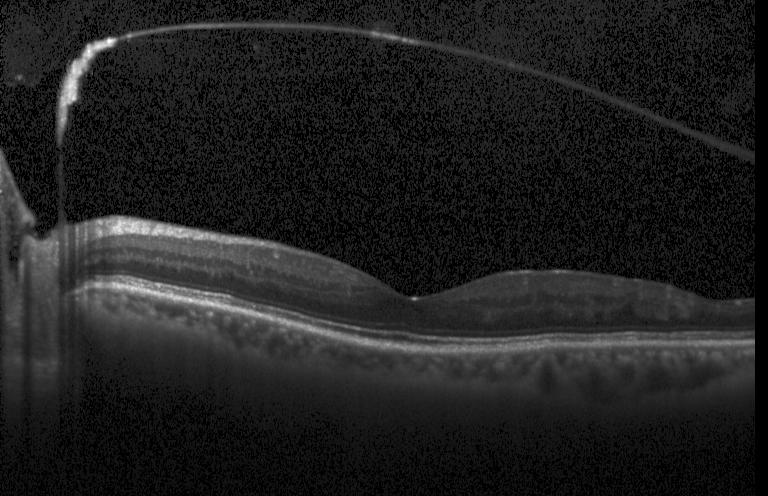

Finding: no choroidal neovascularization, diabetic macular edema, or drusen.